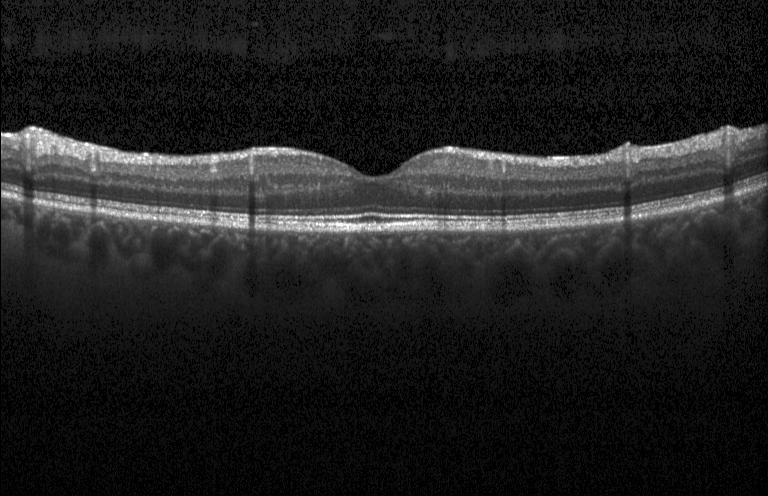 Acquired on a Heidelberg Spectralis, optical coherence tomography B-scan. No CNV, DME, or drusen.